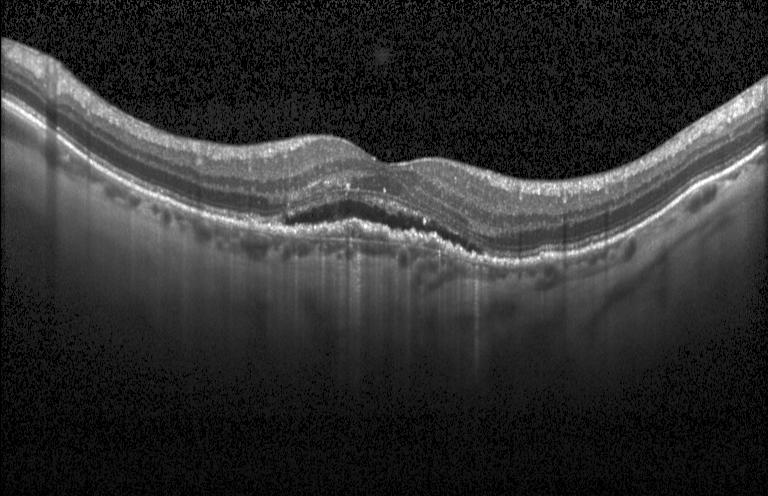

Diagnosis: CNV.